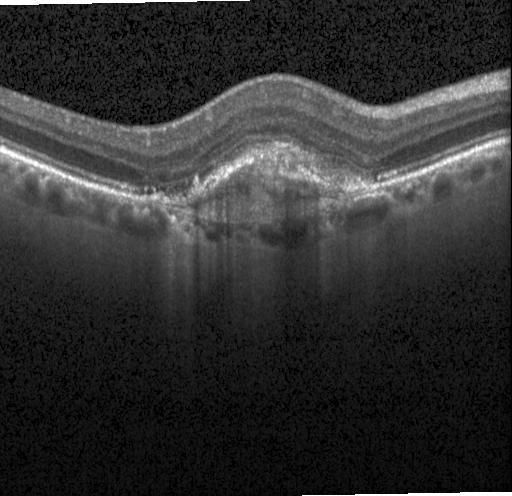
This B-scan demonstrates choroidal neovascularization.